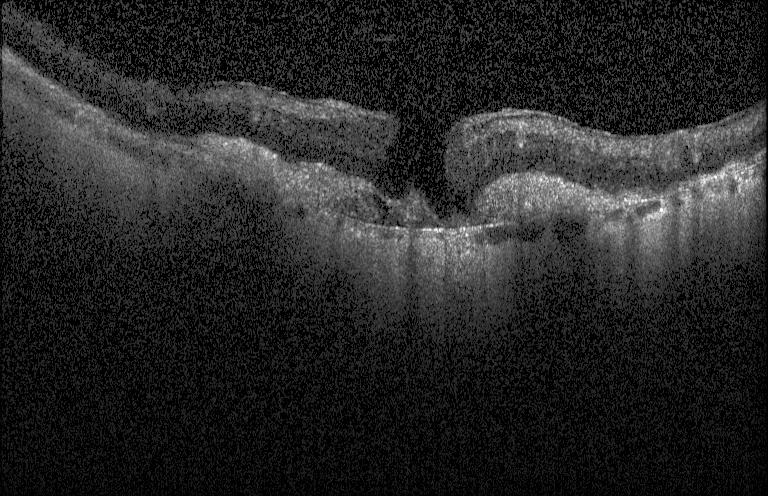

Impression: choroidal neovascularization.